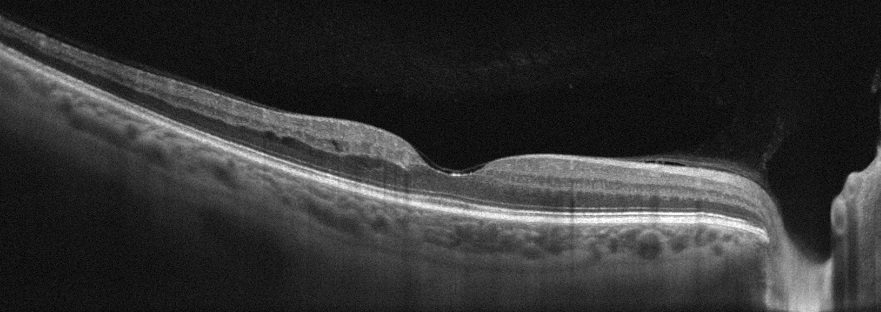

Retinal OCT B-scan — The scan shows diabetic macular edema (DME).